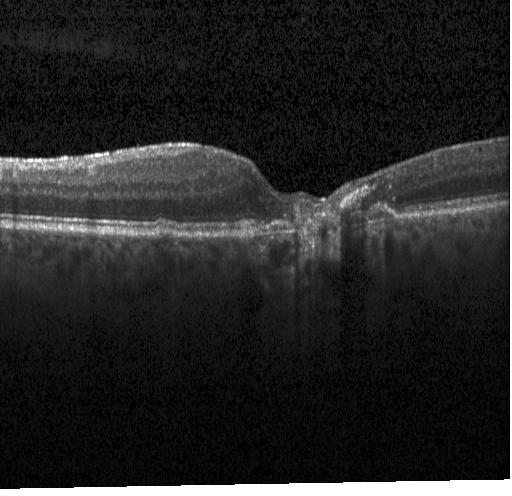
Optical coherence tomography scan. Impression: CNV.